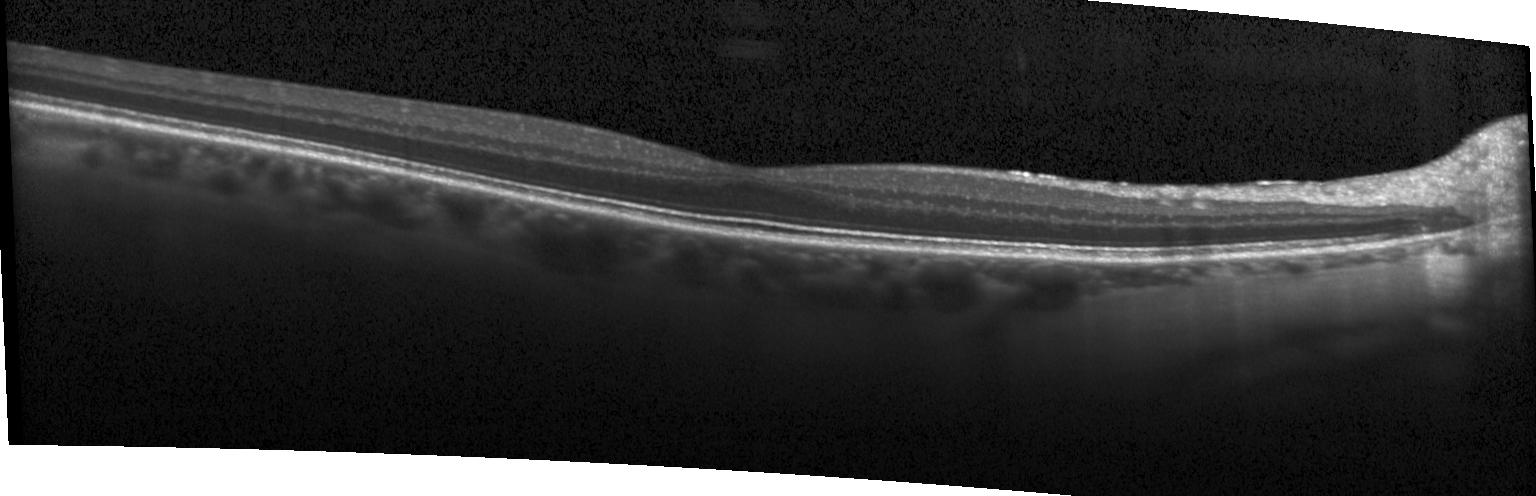
Centered on the fovea, OCT B-scan, spectral-domain OCT.
Finding: no evidence of choroidal neovascularization, diabetic macular edema, or drusen.